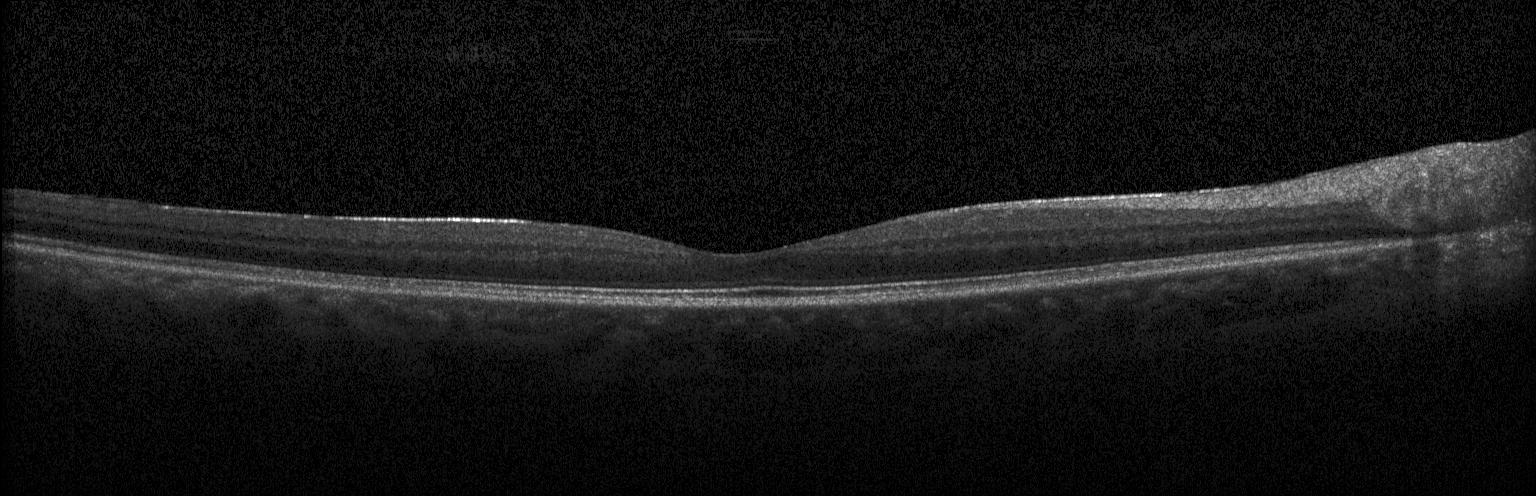 OCT finding: neither choroidal neovascularization, diabetic macular edema, nor drusen.